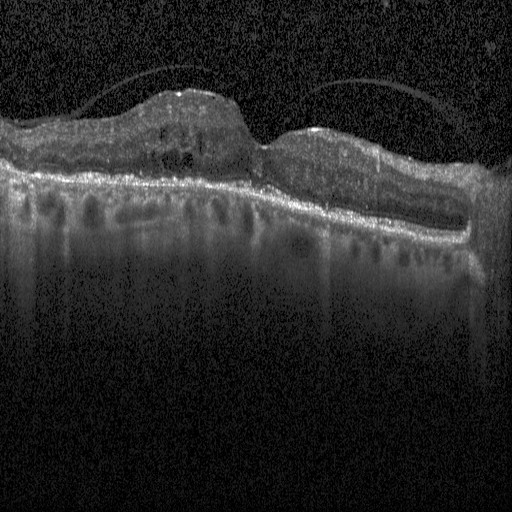

SD-OCT. Macular scan. Acquired on a Heidelberg Spectralis. Optical coherence tomography scan.
Diagnosis: DME.